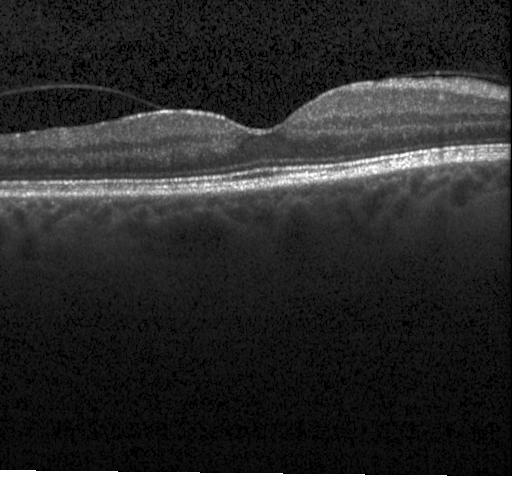 Spectral-domain OCT · through the macula · retinal OCT cross-section.
Impression: no choroidal neovascularization, diabetic macular edema, or drusen.